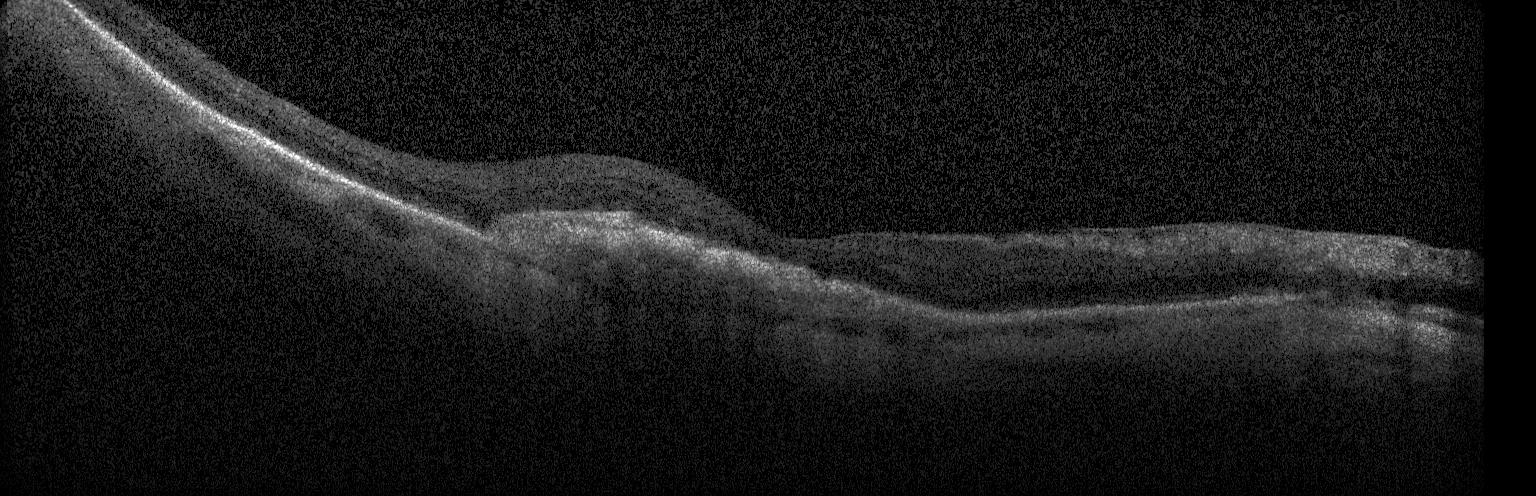

OCT line scan — Assessment: a choroidal neovascular membrane.